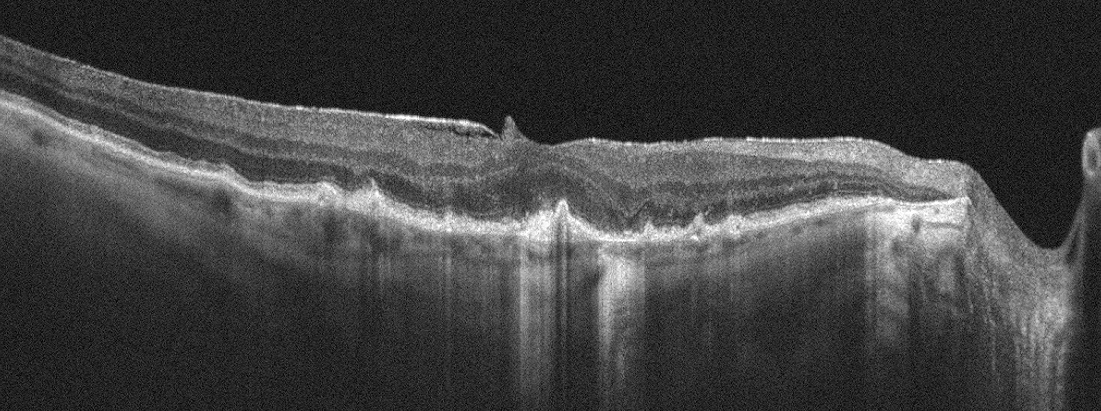

Through the macula; OCT line scan
Impression: age-related macular degeneration.